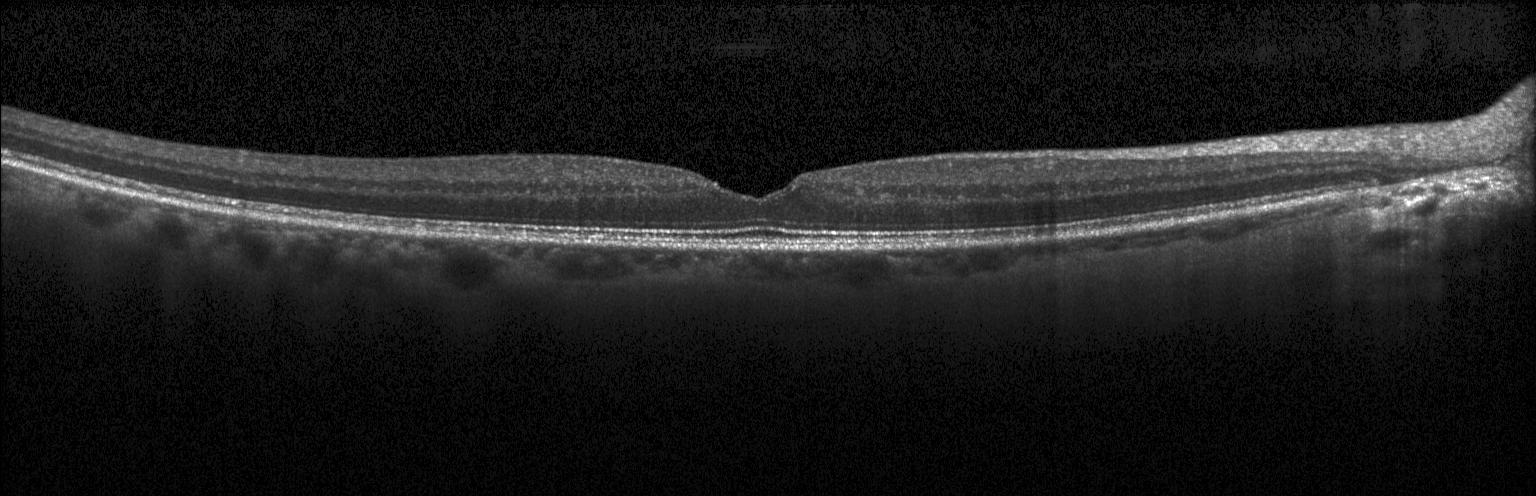 Macular OCT demonstrating neither CNV, DME, nor drusen.